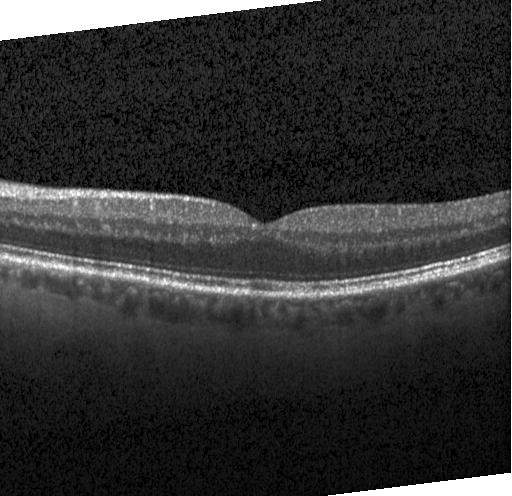 Spectral-domain optical coherence tomography, retinal OCT B-scan, fovea-centered
The scan shows no evidence of choroidal neovascularization, diabetic macular edema, or drusen.